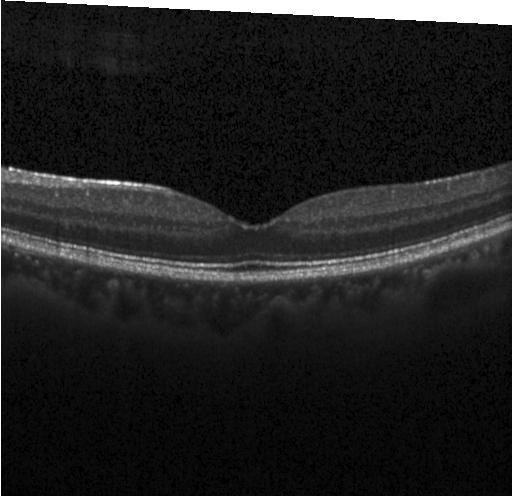
No choroidal neovascularization, diabetic macular edema, or drusen.